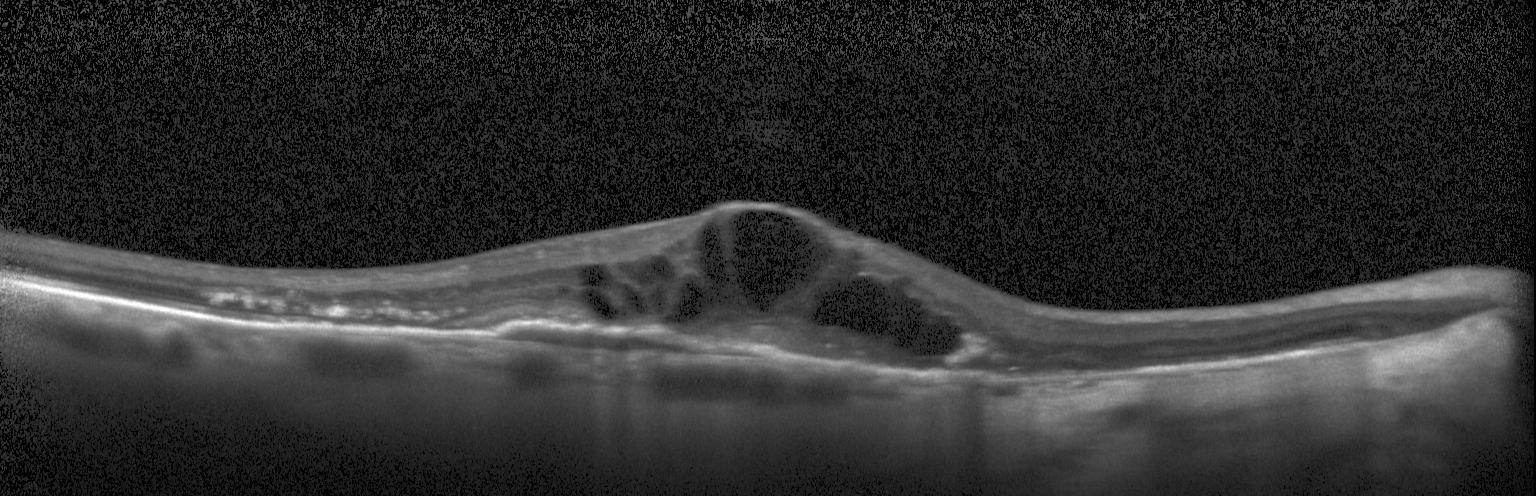 Retinal OCT cross-section showing a choroidal neovascular membrane.